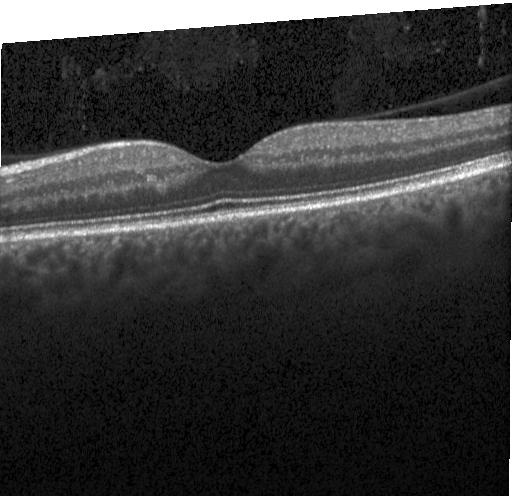 OCT B-scan. Finding: no choroidal neovascularization, diabetic macular edema, or drusen.